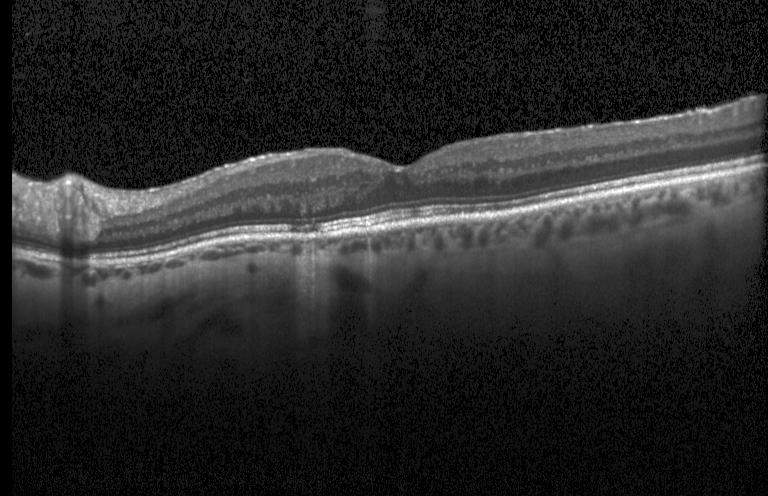

Macular OCT: neither CNV, DME, nor drusen.